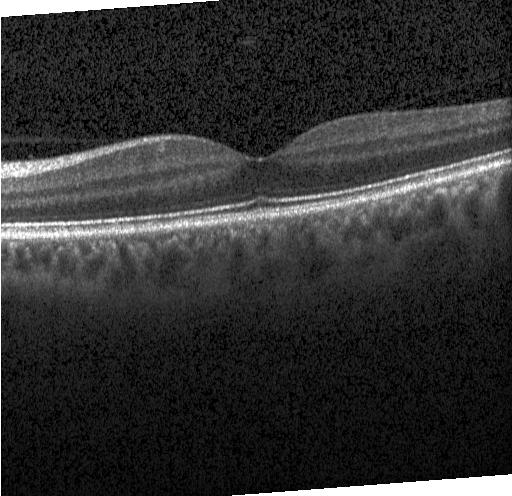

OCT line scan, spectral-domain optical coherence tomography, Heidelberg Spectralis OCT system.
Finding: no CNV, DME, or drusen.